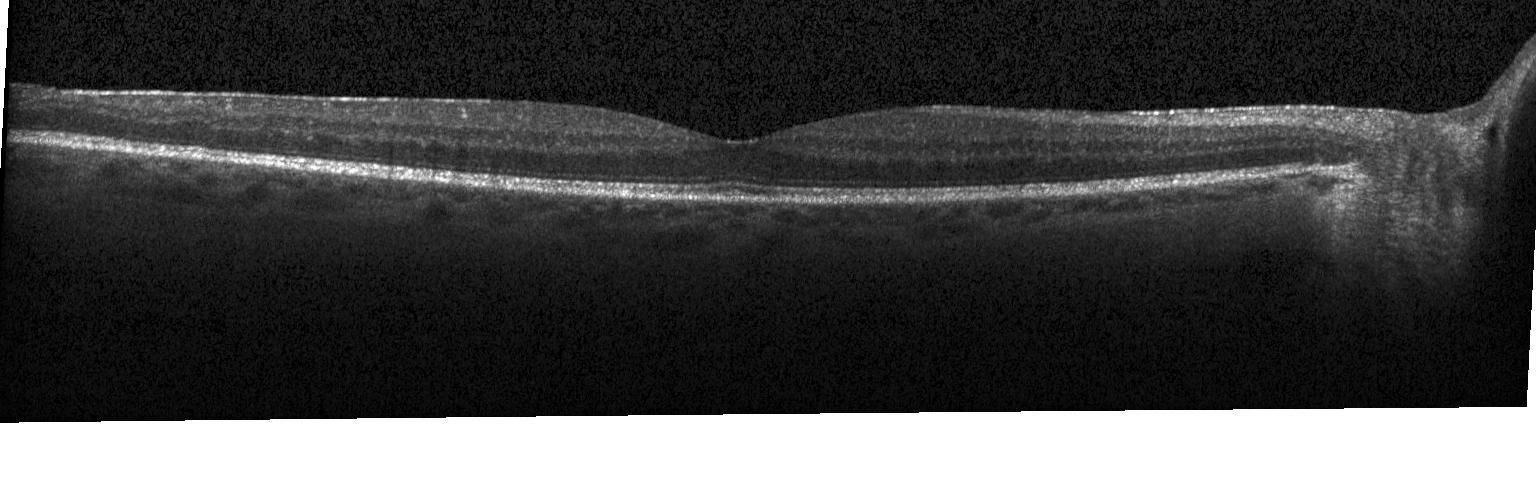

Optical coherence tomography scan · Heidelberg Spectralis OCT system.
Diagnosis: no evidence of choroidal neovascularization, diabetic macular edema, or drusen.